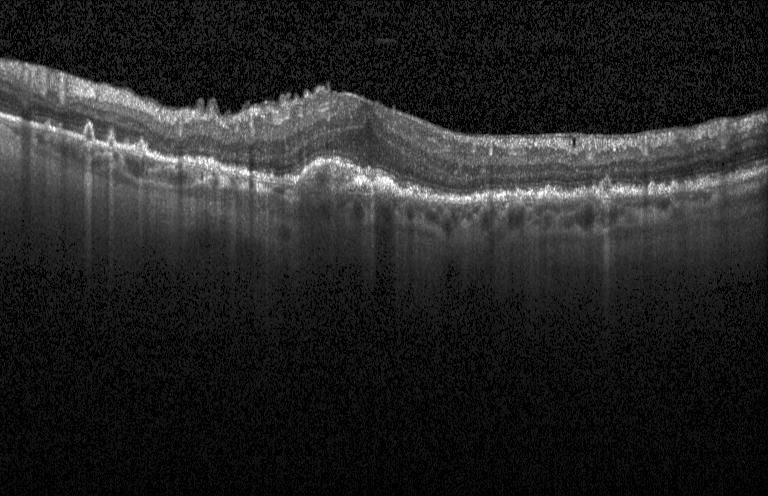 Optical coherence tomography B-scan.
This B-scan demonstrates a choroidal neovascular membrane.